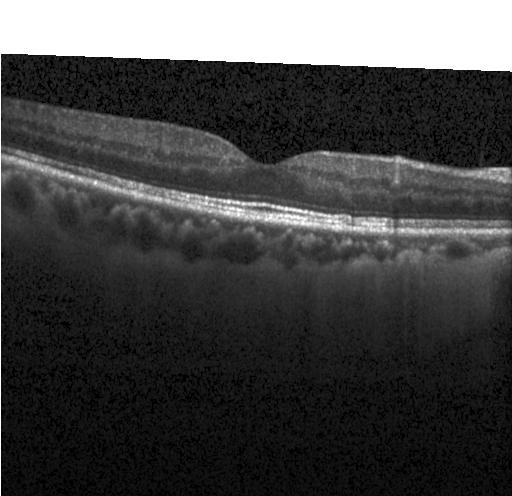
Impression: no evidence of choroidal neovascularization, diabetic macular edema, or drusen.